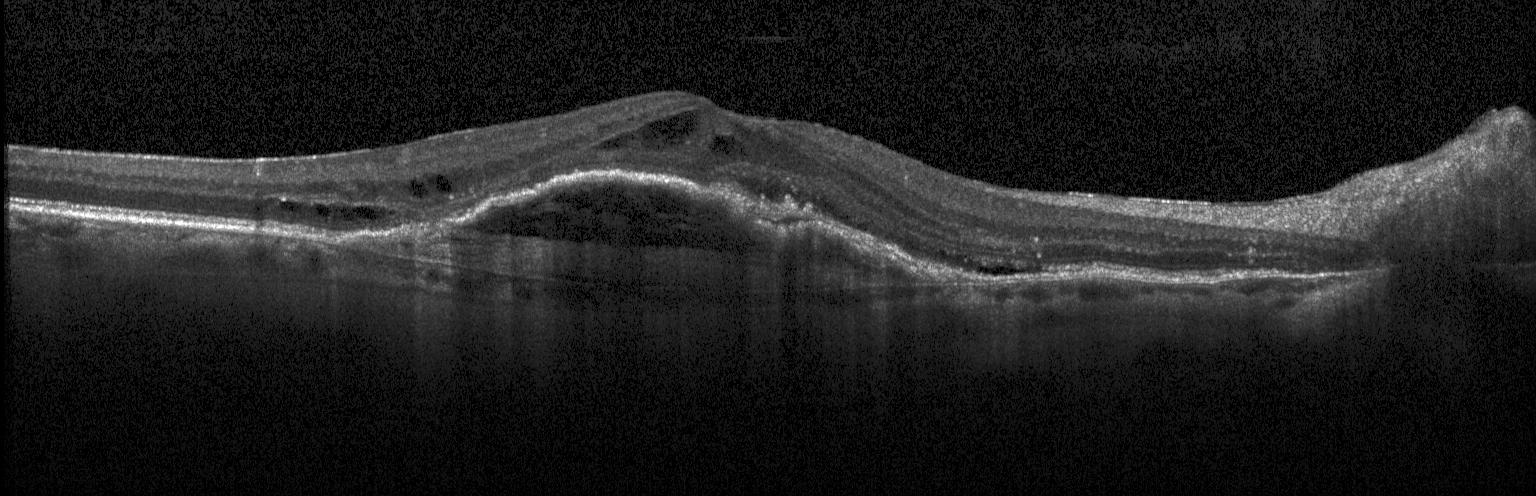
Retinal OCT cross-section. Spectral-domain optical coherence tomography. Instrument: Heidelberg Spectralis. Finding: choroidal neovascularization (CNV).